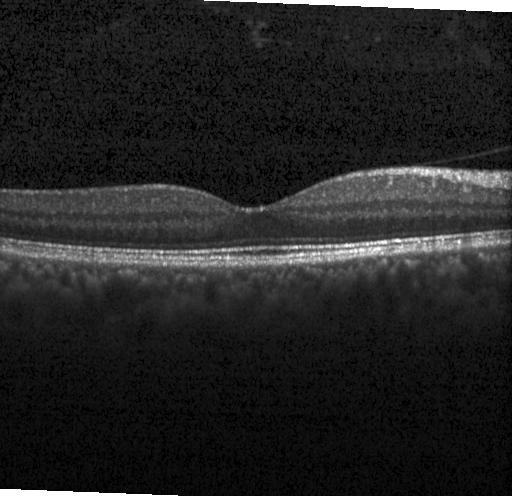 The scan shows neither choroidal neovascularization, diabetic macular edema, nor drusen.